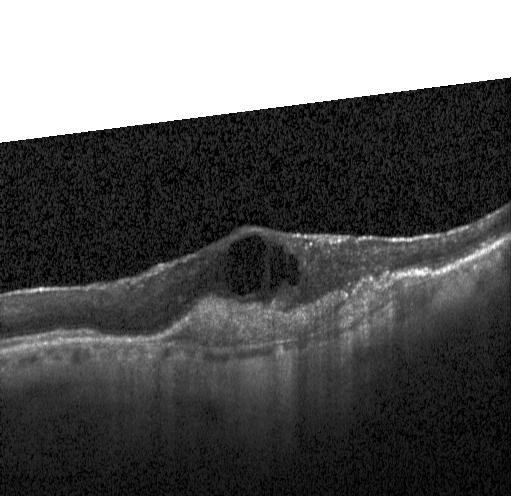

Heidelberg Spectralis OCT system; retinal OCT B-scan; through the macula; spectral-domain OCT — Diagnosis: a choroidal neovascular membrane.